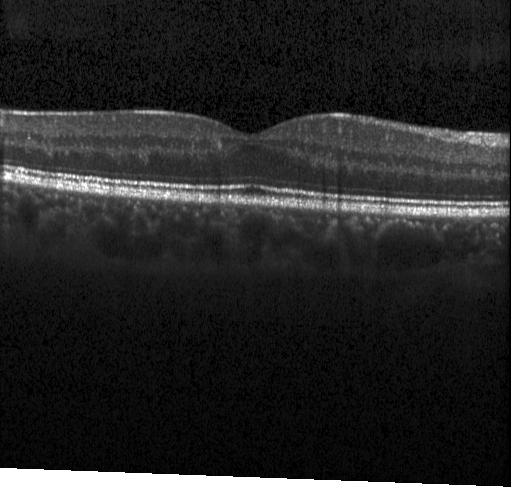

OCT line scan — Macular OCT: no CNV, DME, or drusen.